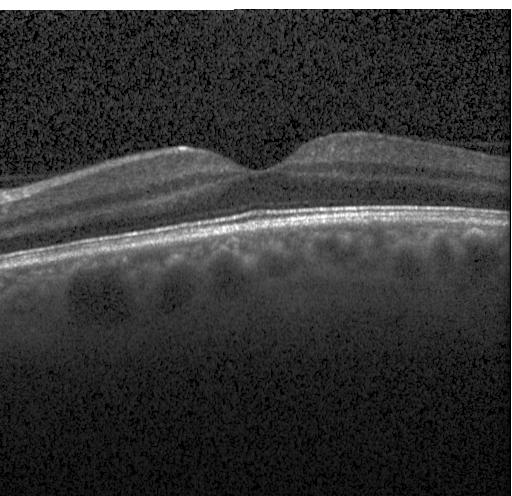
Retinal OCT cross-section; horizontal scan through the fovea; spectral-domain OCT
Finding: neither choroidal neovascularization, diabetic macular edema, nor drusen.